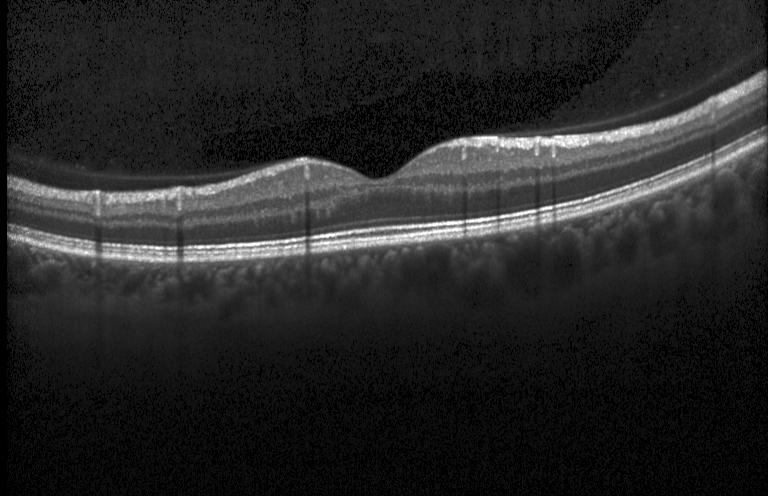 Optical coherence tomography scan · spectral-domain optical coherence tomography.
Dx: neither choroidal neovascularization, diabetic macular edema, nor drusen.